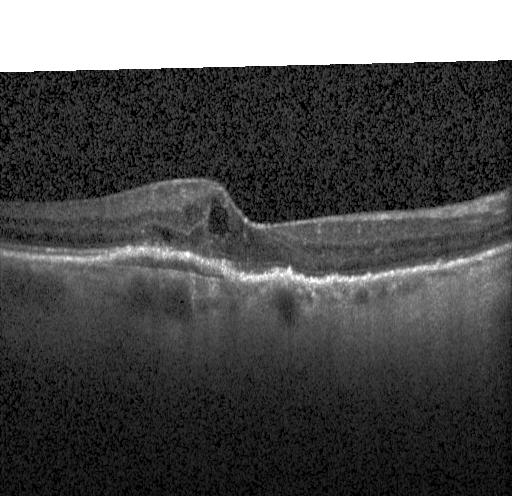
OCT B-scan. The scan shows a choroidal neovascular membrane.